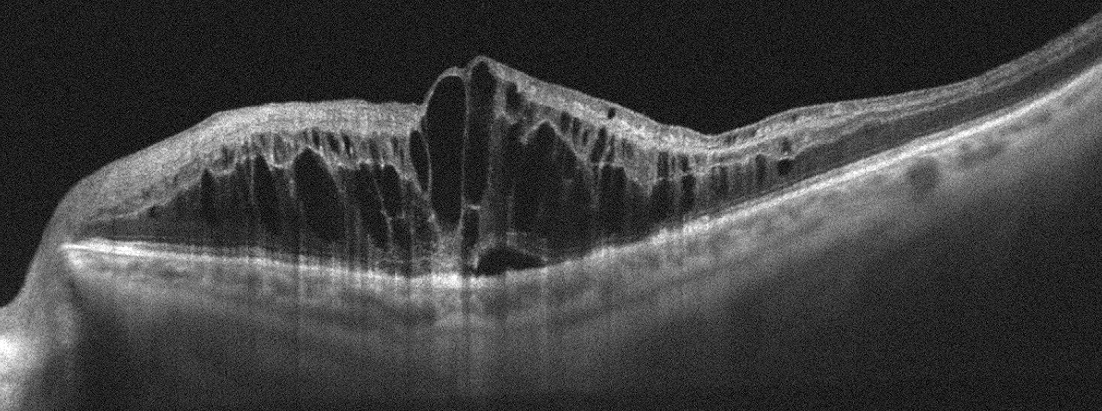

OCT B-scan. Optovue Avanti RTVue XR. Fovea-centered. Macular OCT: RVO.